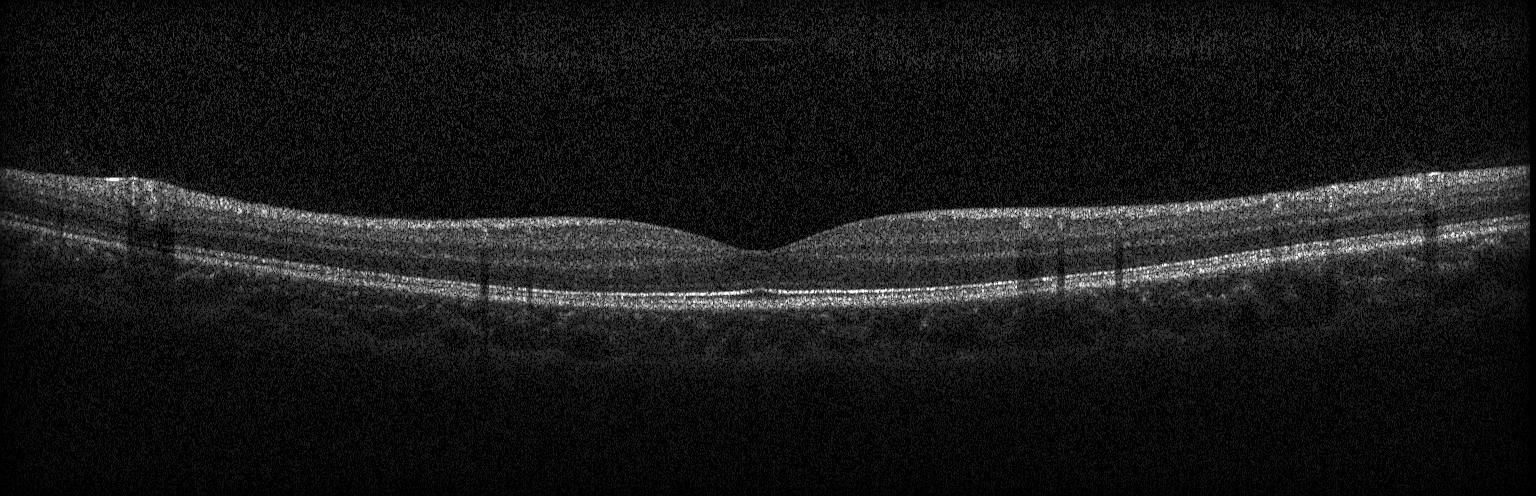 OCT scan showing no choroidal neovascularization, no diabetic macular edema, and no drusen.